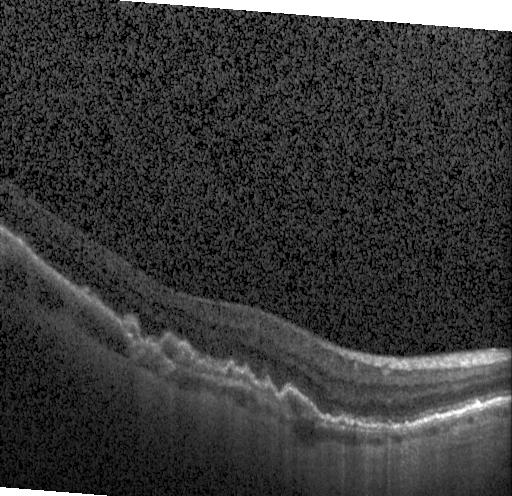
Macular scan, SD-OCT, OCT B-scan, Heidelberg Spectralis. Finding: a choroidal neovascular membrane.